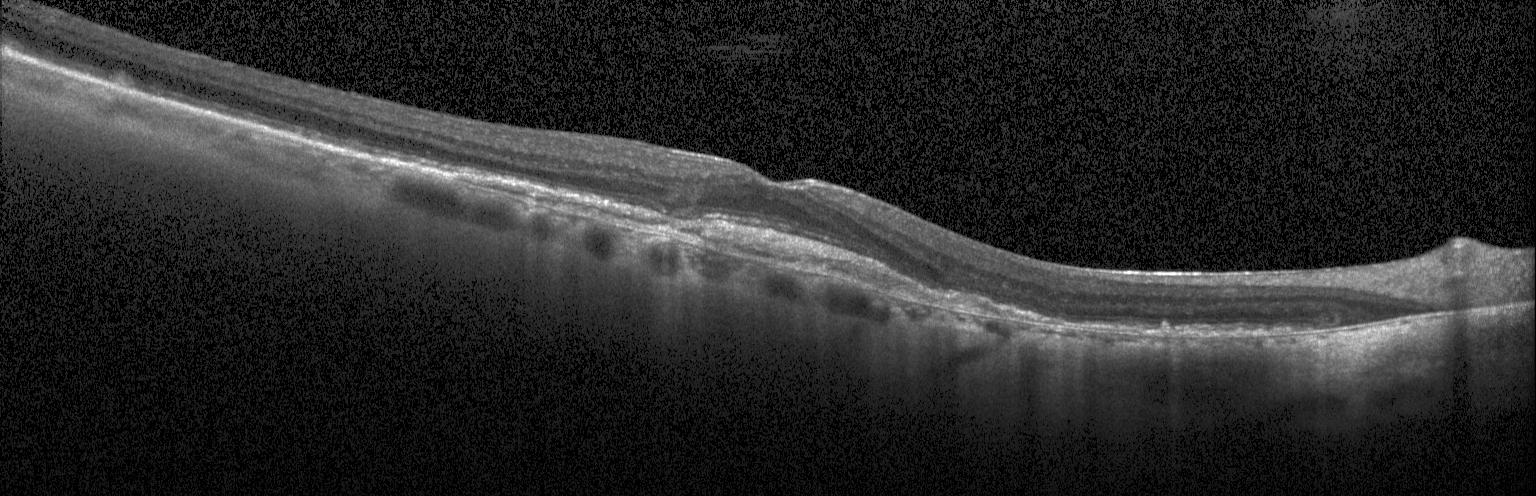
Optical coherence tomography B-scan; SD-OCT.
Impression: choroidal neovascularization (CNV).